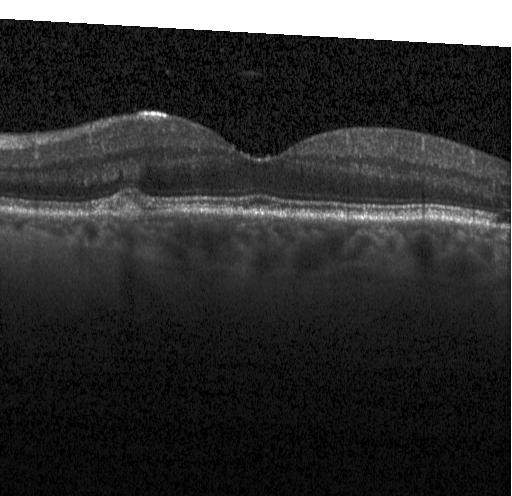 OCT finding: sub-RPE drusenoid deposits.